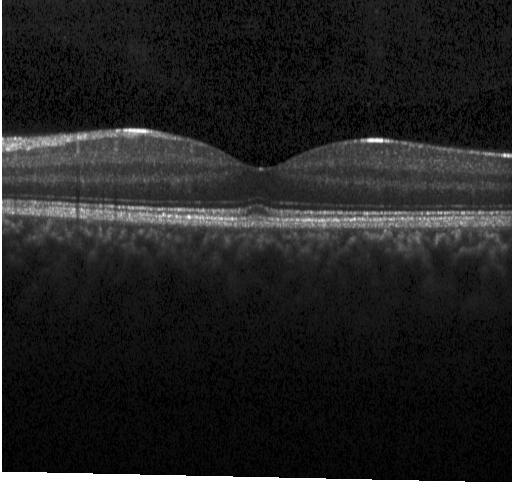
Impression: no CNV, no DME, and no drusen.